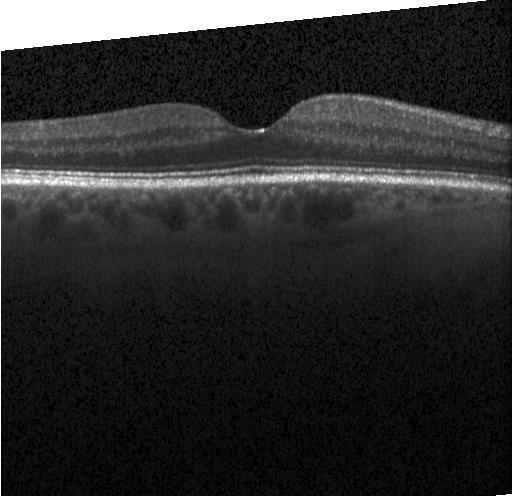
Diagnosis: no choroidal neovascularization, diabetic macular edema, or drusen.